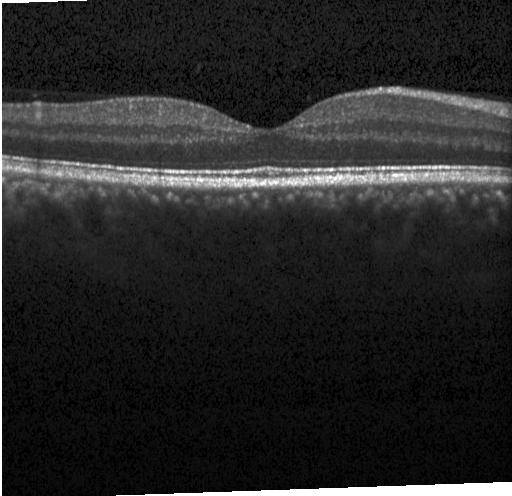

OCT line scan
Finding: no choroidal neovascularization, diabetic macular edema, or drusen.